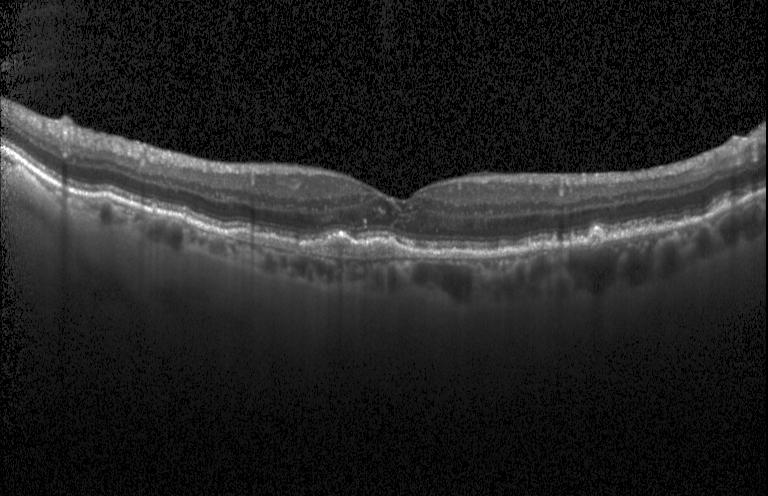 Retinal OCT B-scan
A choroidal neovascular membrane.